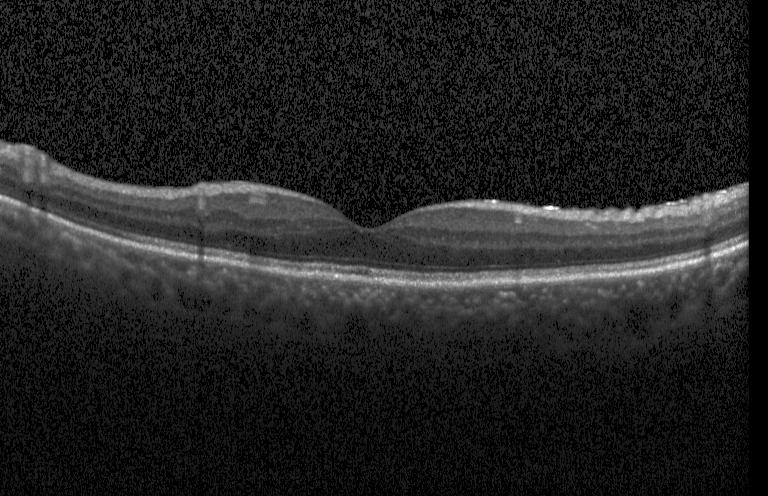

OCT line scan.
Assessment: no choroidal neovascularization, no diabetic macular edema, and no drusen.